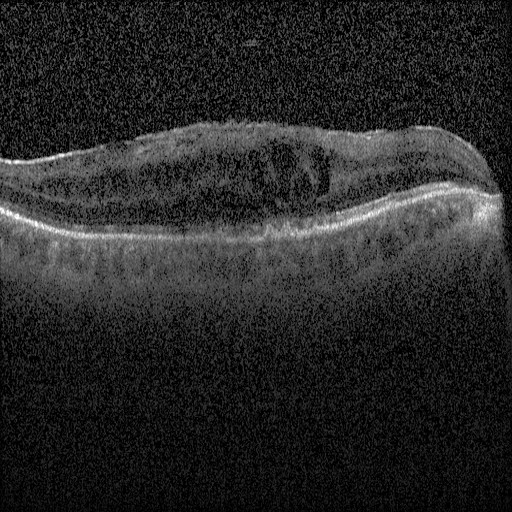 Retinal OCT B-scan — Diagnosis: diabetic macular edema (DME).